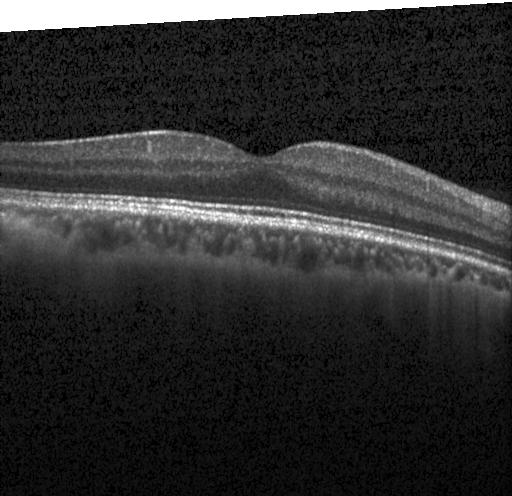 Acquired on a Heidelberg Spectralis. Spectral-domain OCT. OCT B-scan. Horizontal scan through the fovea — This B-scan demonstrates no choroidal neovascularization, diabetic macular edema, or drusen.